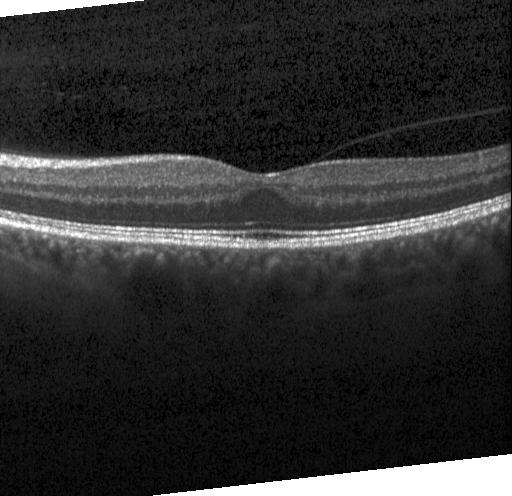
Impression: no evidence of choroidal neovascularization, diabetic macular edema, or drusen.